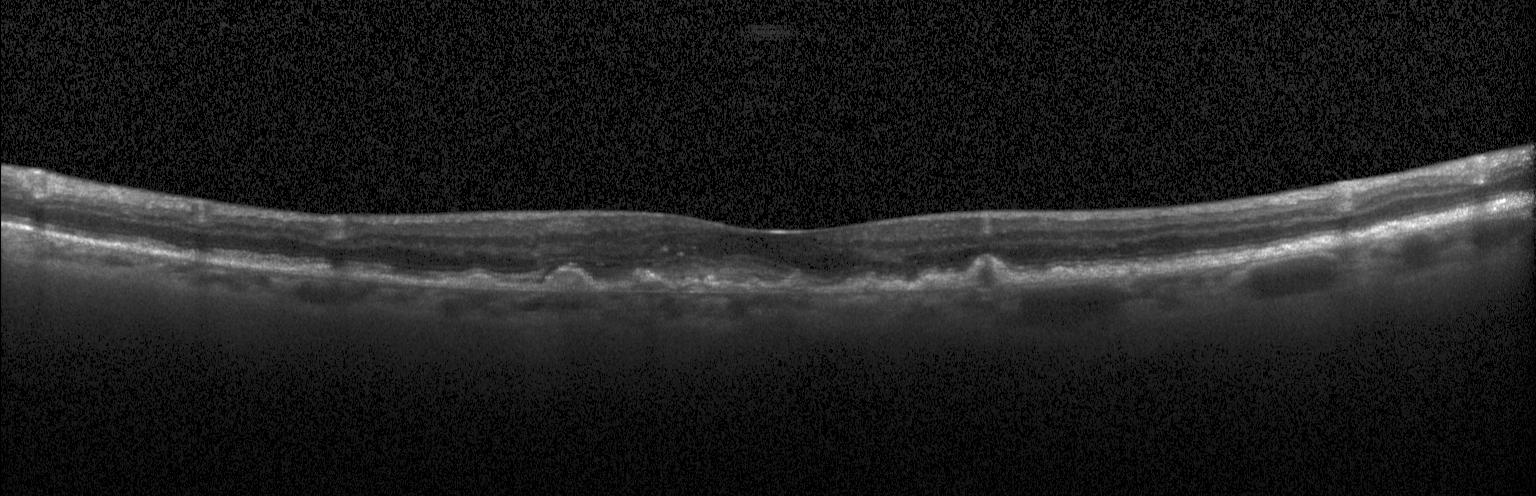

Impression: a choroidal neovascular membrane.